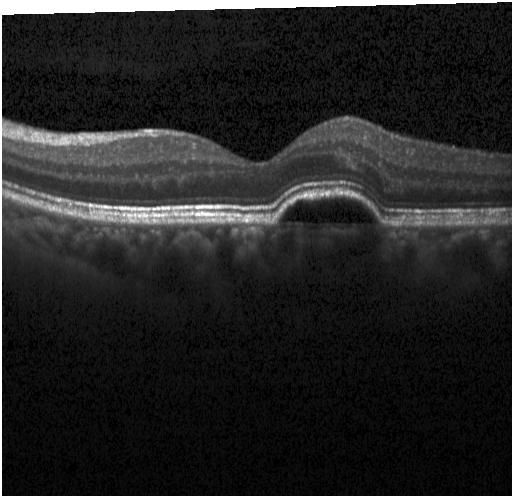
Centered on the fovea. Optical coherence tomography scan. Dx: CNV.